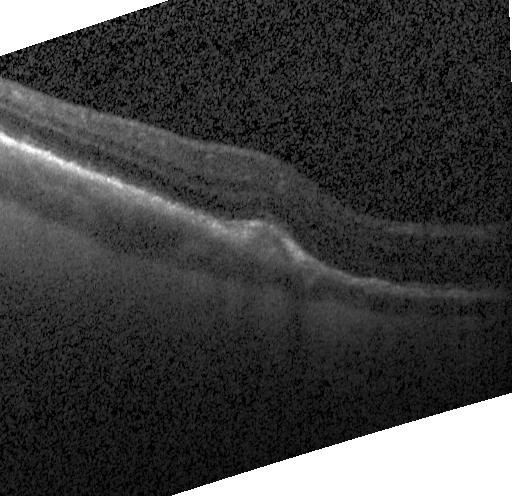

Heidelberg Spectralis, retinal OCT B-scan — Finding: CNV.